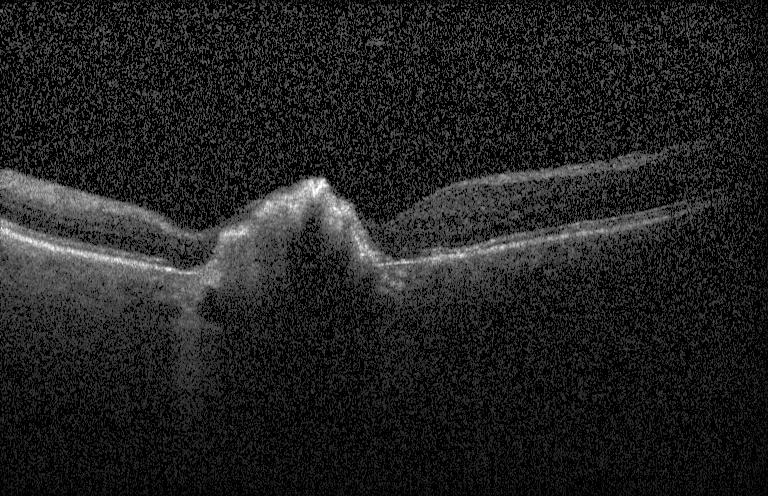
Diagnosis: a choroidal neovascular membrane.